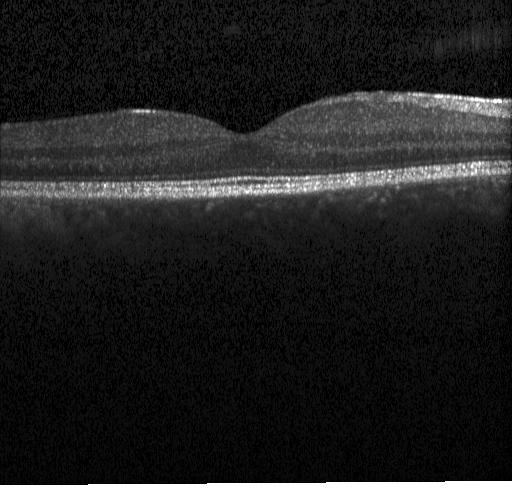

SD-OCT, OCT line scan. Finding: no choroidal neovascularization, no diabetic macular edema, and no drusen.